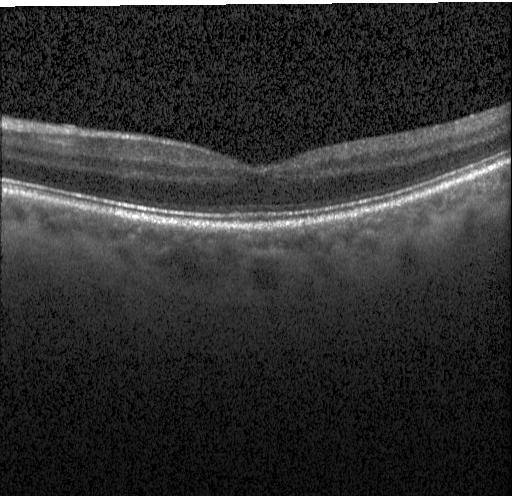

OCT scan showing no choroidal neovascularization, diabetic macular edema, or drusen.